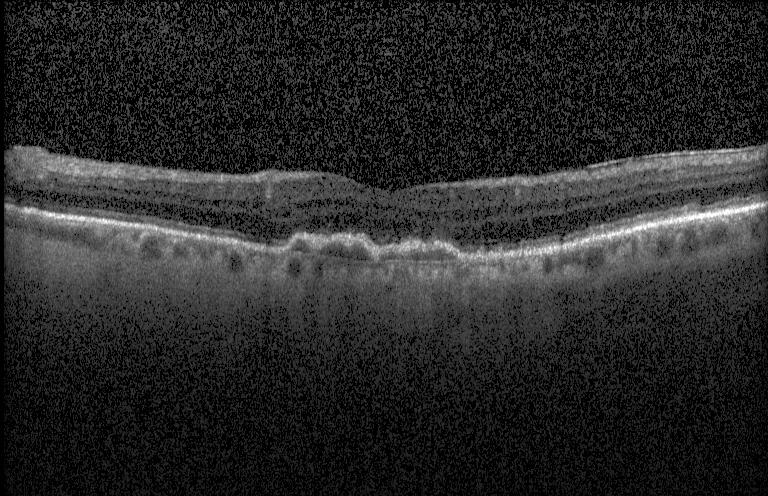

Acquired on a Heidelberg Spectralis, macular scan, spectral-domain OCT, OCT B-scan.
Diagnosis: CNV.